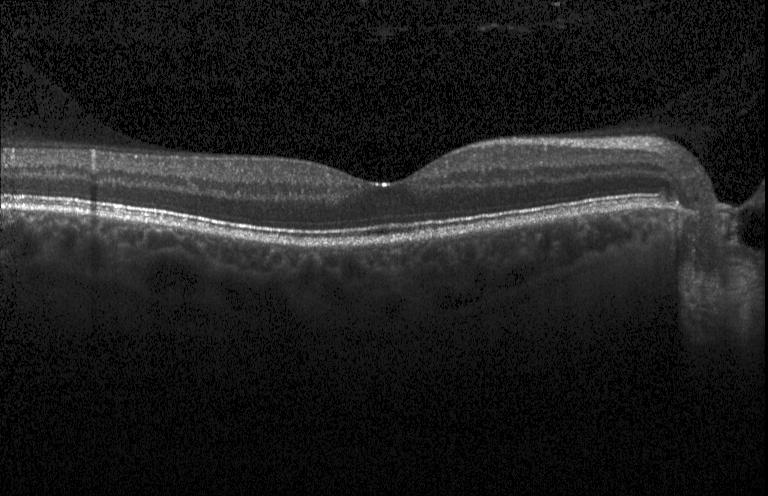
Diagnosis: no evidence of choroidal neovascularization, diabetic macular edema, or drusen.